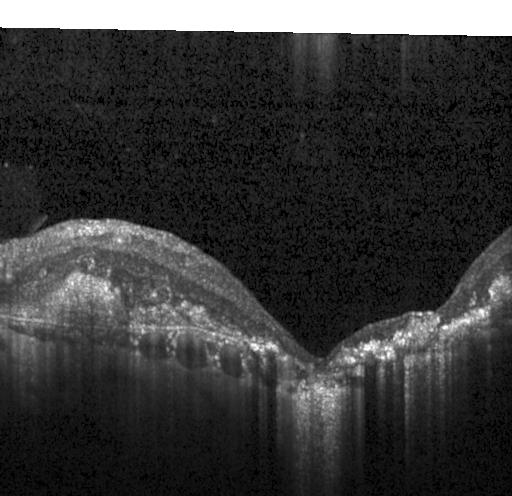

Spectral-domain optical coherence tomography, centered on the fovea, OCT B-scan, Heidelberg Spectralis OCT system
Diagnosis: a choroidal neovascular membrane.